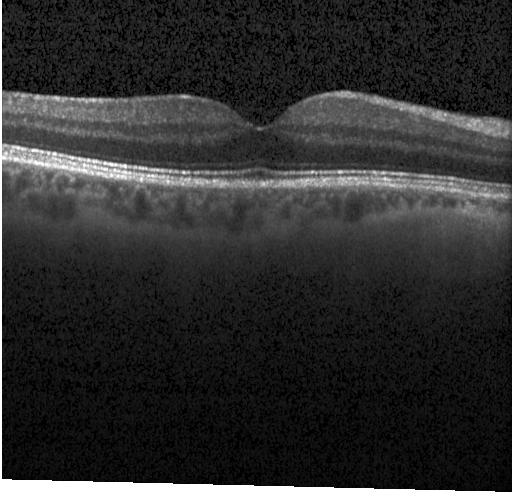 No choroidal neovascularization, diabetic macular edema, or drusen.